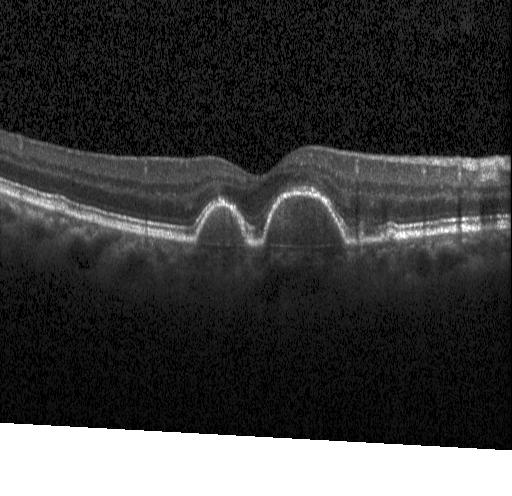

This B-scan demonstrates sub-RPE drusenoid deposits.